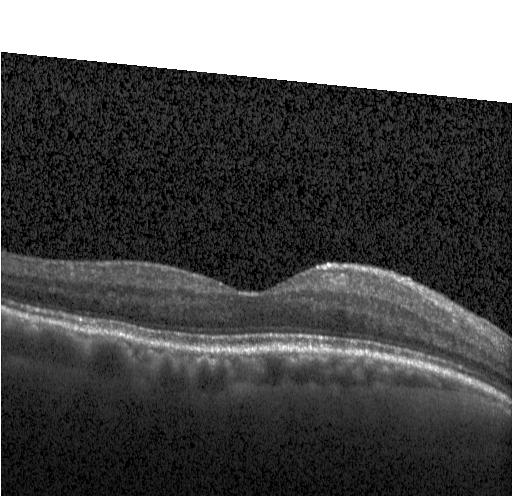 Heidelberg Spectralis OCT system · OCT line scan · spectral-domain optical coherence tomography · centered on the fovea
Macular OCT: no choroidal neovascularization, no diabetic macular edema, and no drusen.